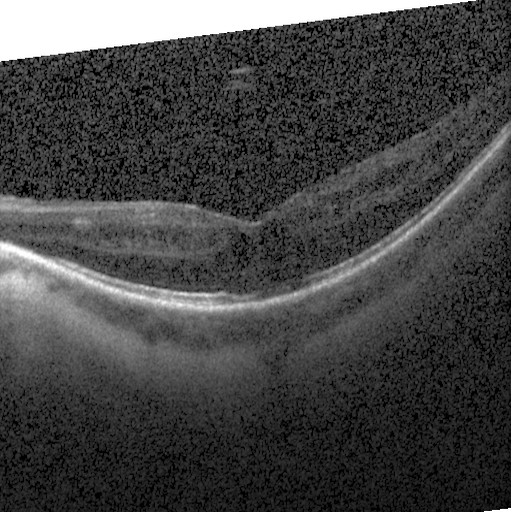
OCT line scan.
Impression: DME.